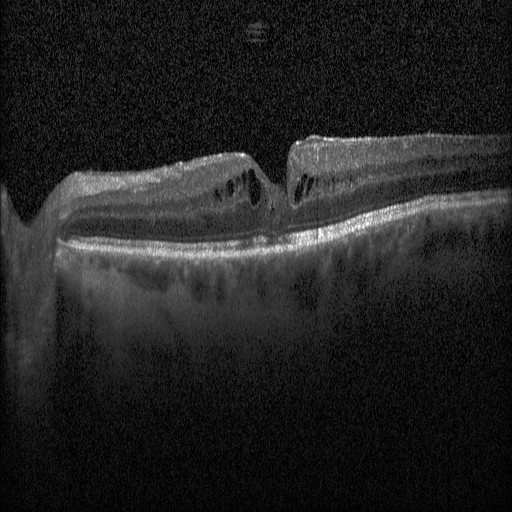 Retinal OCT B-scan. Spectral-domain OCT. Heidelberg Spectralis OCT system
The scan shows diabetic macular edema.